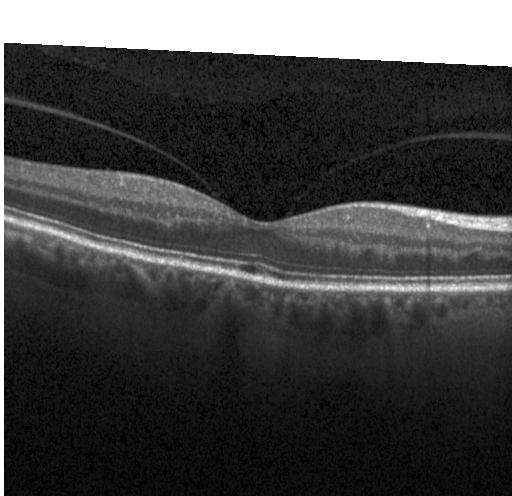
Finding: neither choroidal neovascularization, diabetic macular edema, nor drusen.